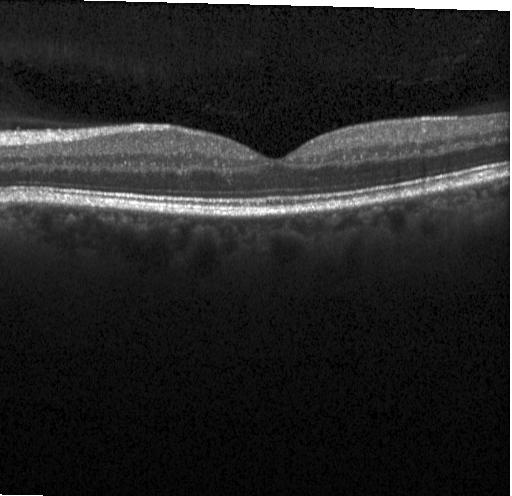

Macular scan · instrument: Heidelberg Spectralis · OCT line scan
Dx: no choroidal neovascularization, diabetic macular edema, or drusen.